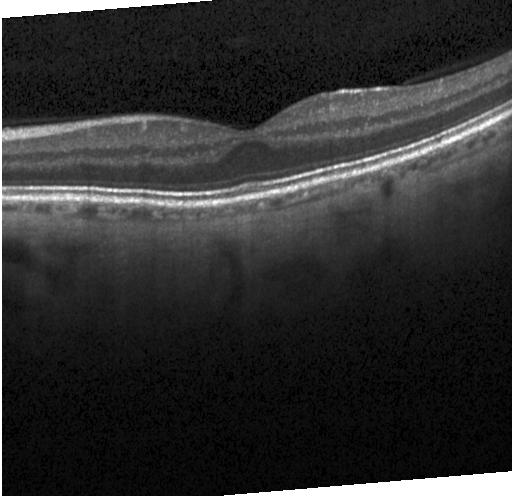
Optical coherence tomography scan. Impression: no choroidal neovascularization, no diabetic macular edema, and no drusen.